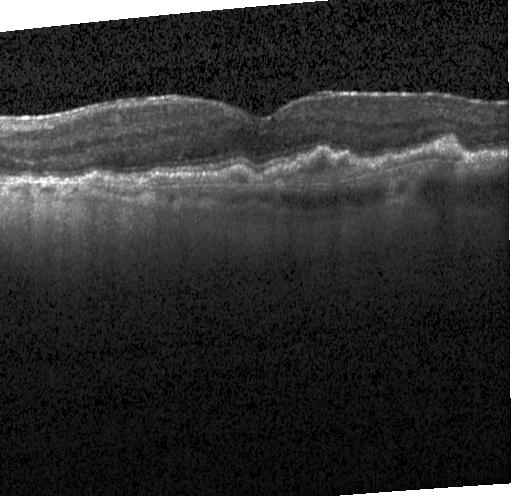 Optical coherence tomography B-scan · Heidelberg Spectralis OCT system.
Macular OCT: CNV.